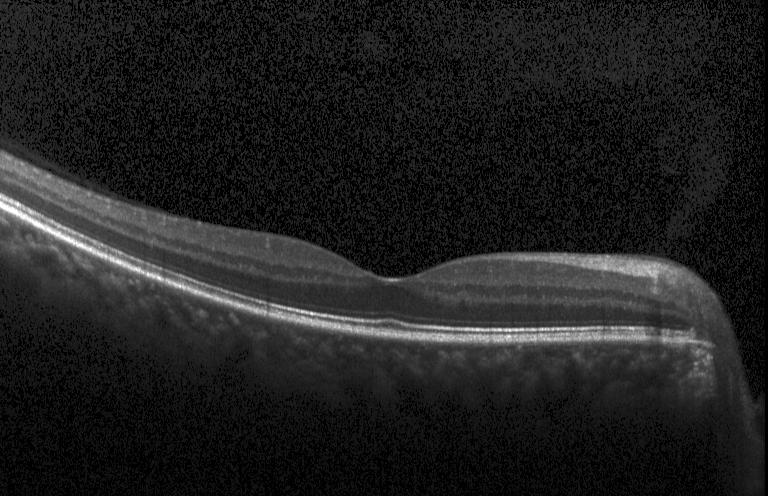
Optical coherence tomography scan; horizontal scan through the fovea; Heidelberg Spectralis OCT system
Finding: no evidence of choroidal neovascularization, diabetic macular edema, or drusen.